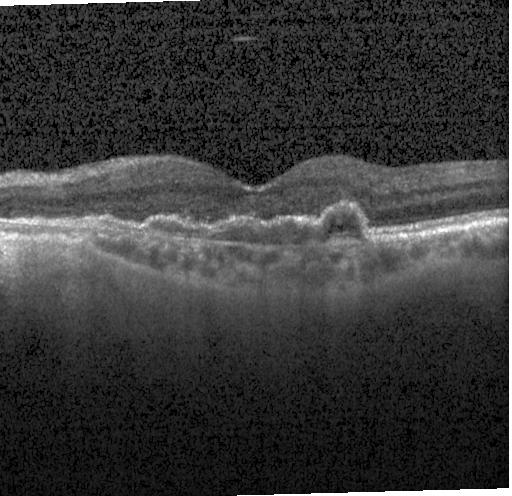

Dx: CNV.